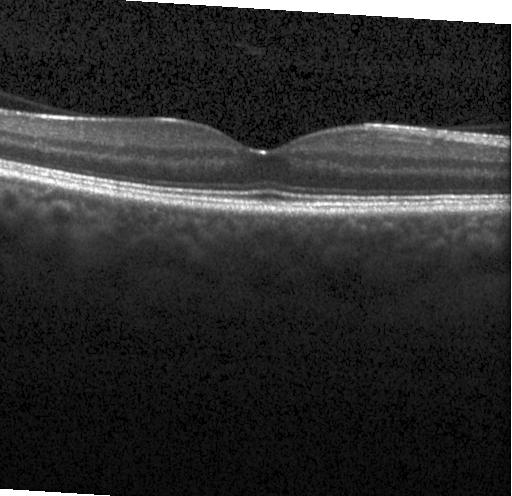
Spectral-domain OCT; acquired on a Heidelberg Spectralis; optical coherence tomography scan; horizontal scan through the fovea. The scan shows no choroidal neovascularization, no diabetic macular edema, and no drusen.